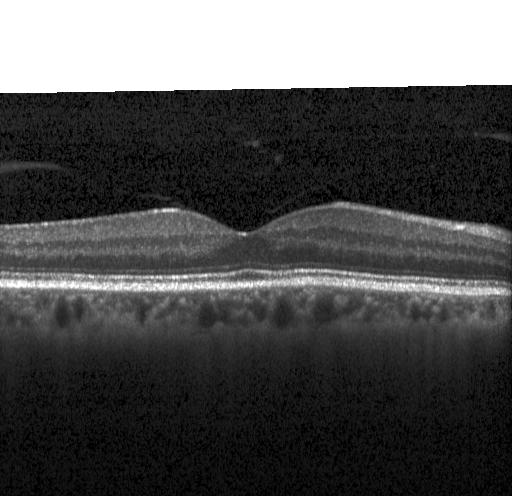
Heidelberg Spectralis, optical coherence tomography scan, horizontal scan through the fovea, spectral-domain OCT
Finding: no evidence of CNV, DME, or drusen.